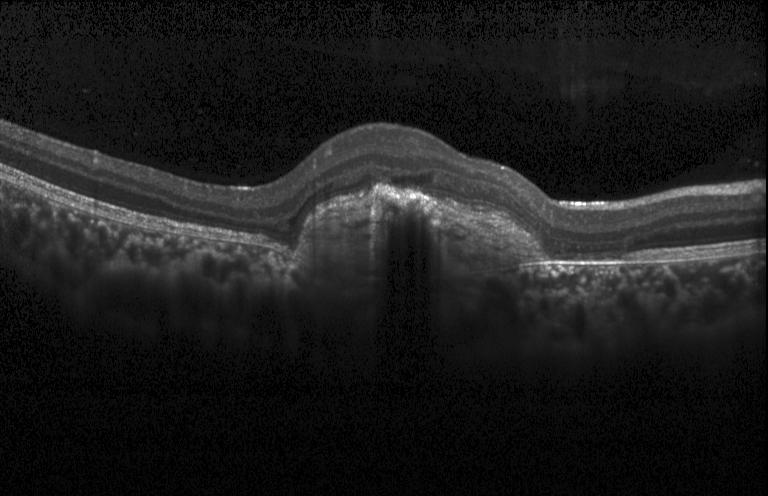 Horizontal scan through the fovea · OCT line scan
Dx: choroidal neovascularization.